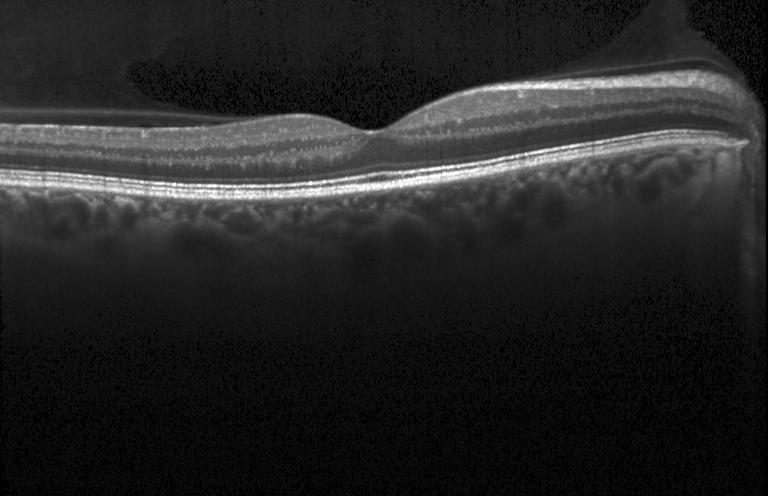 Through the macula · optical coherence tomography scan
This B-scan demonstrates no evidence of choroidal neovascularization, diabetic macular edema, or drusen.